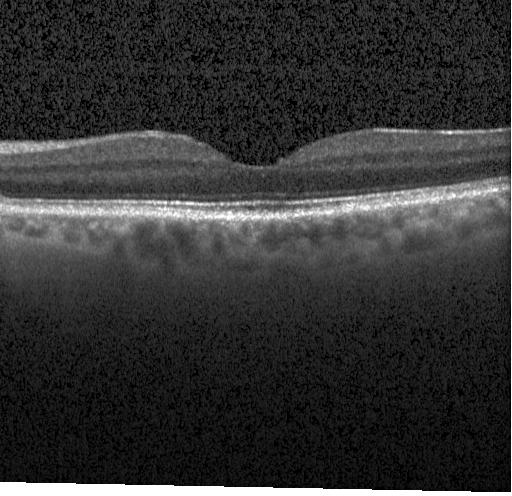
Diagnosis: no choroidal neovascularization, diabetic macular edema, or drusen.